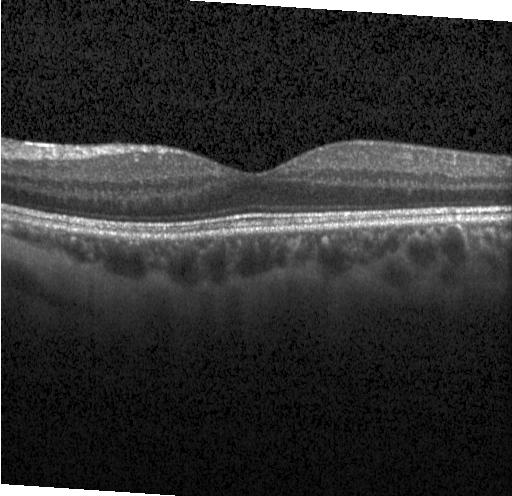
Optical coherence tomography scan.
The scan shows neither choroidal neovascularization, diabetic macular edema, nor drusen.